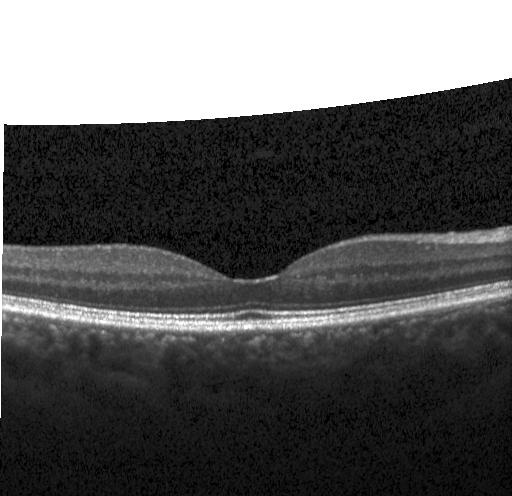 Dx: neither choroidal neovascularization, diabetic macular edema, nor drusen.